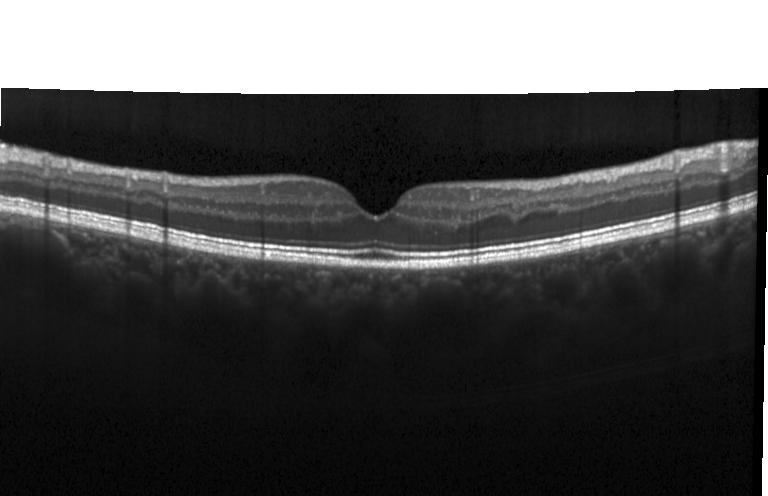
Diagnosis: no CNV, no DME, and no drusen.